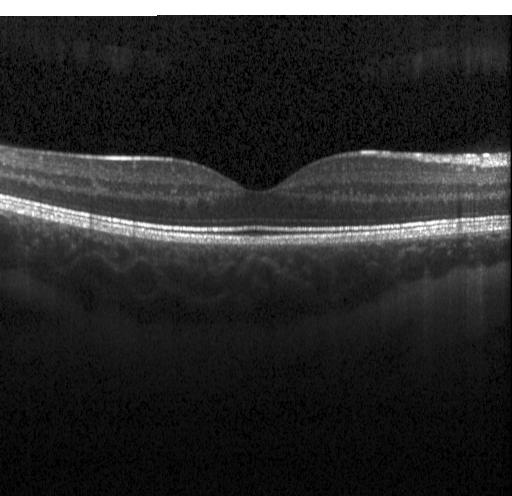

OCT B-scan showing neither choroidal neovascularization, diabetic macular edema, nor drusen.